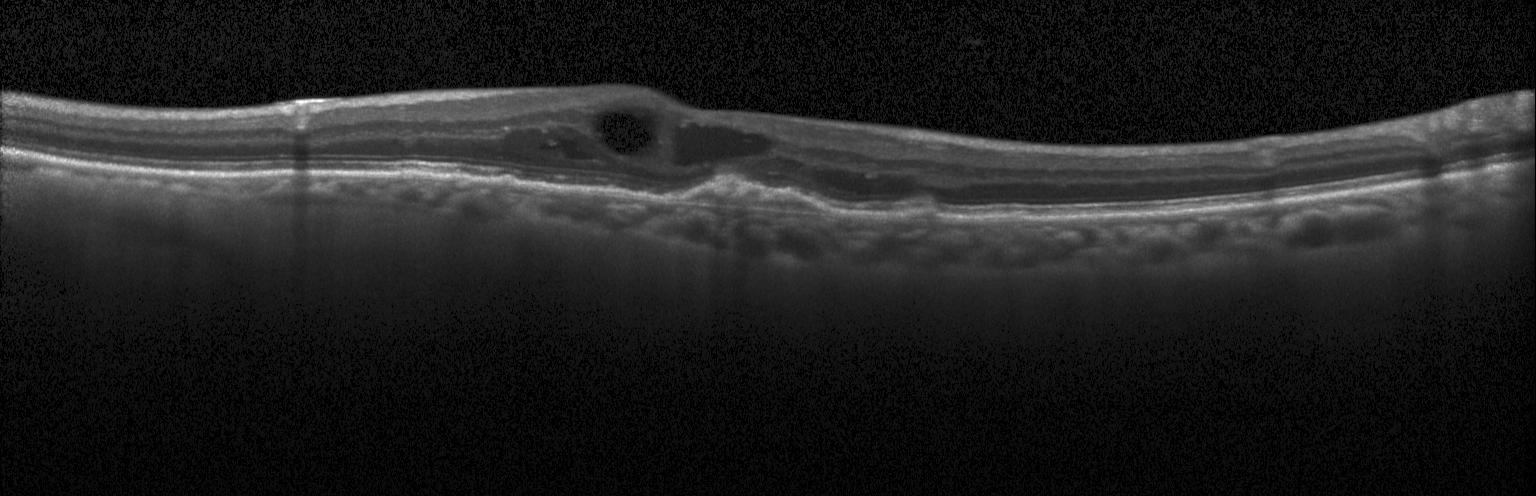
Assessment: choroidal neovascularization (CNV).